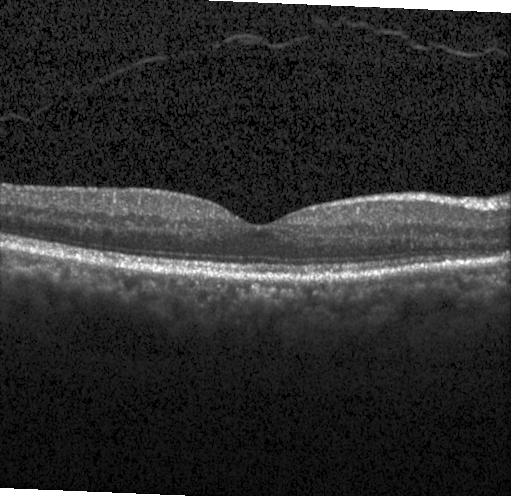

Diagnosis: no evidence of choroidal neovascularization, diabetic macular edema, or drusen.